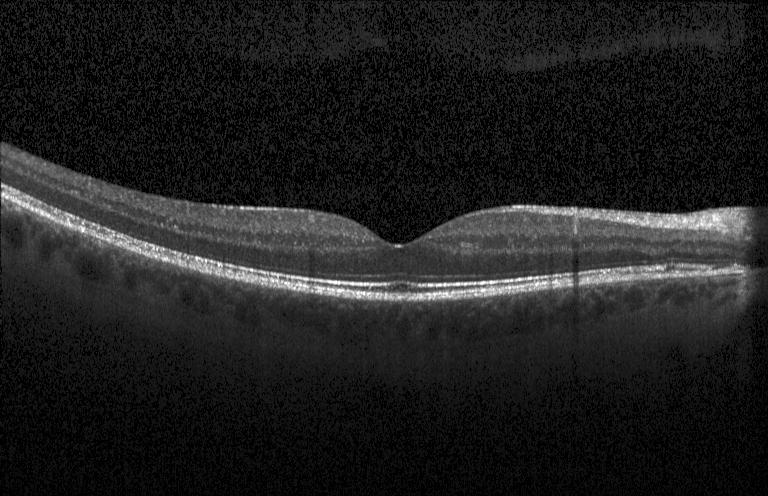
Neither CNV, DME, nor drusen.